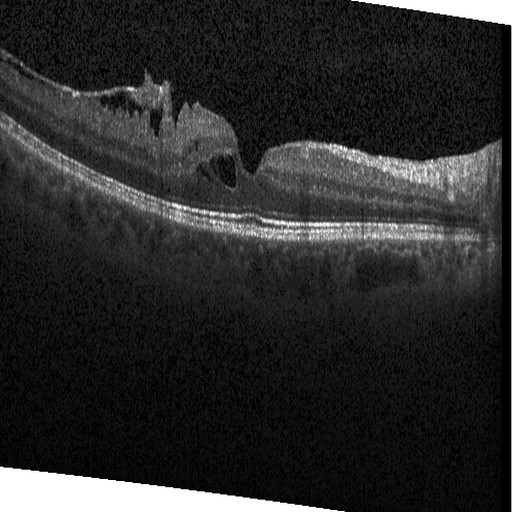

Macular scan, retinal OCT cross-section, spectral-domain optical coherence tomography. Dx: diabetic macular edema.